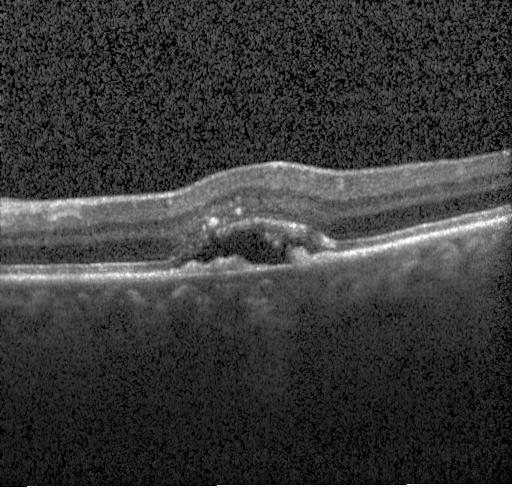
Impression: a choroidal neovascular membrane.